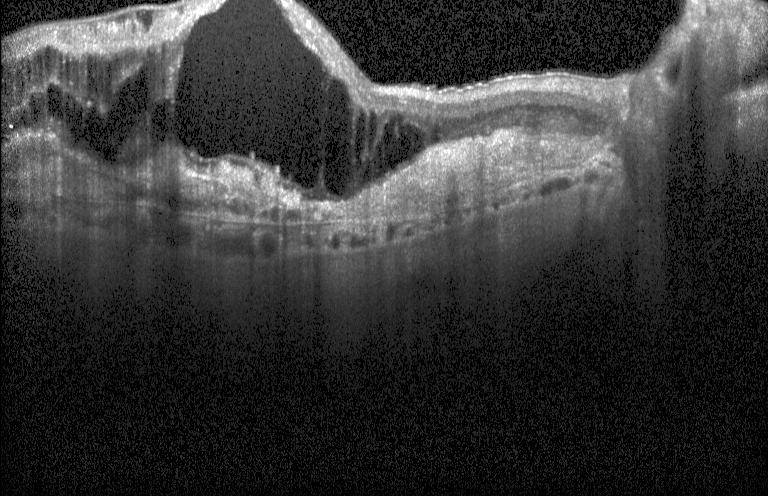
Macular scan. OCT line scan
Finding: a choroidal neovascular membrane.